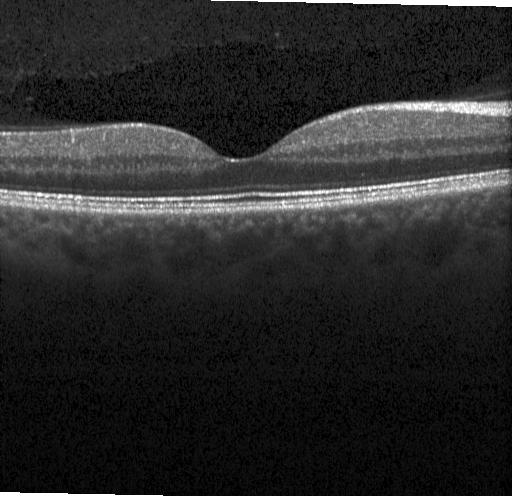

Macular scan. Retinal OCT cross-section. Heidelberg Spectralis. This B-scan demonstrates no evidence of choroidal neovascularization, diabetic macular edema, or drusen.